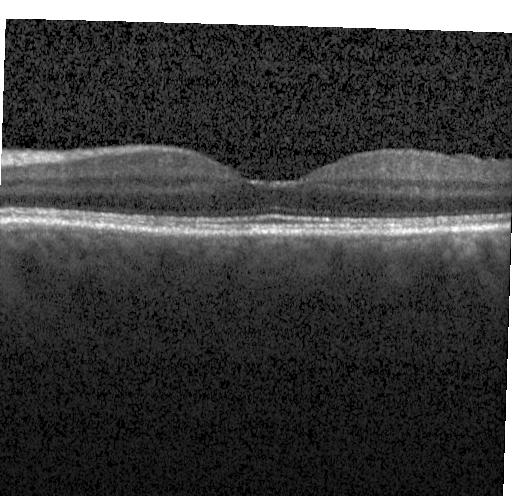 This B-scan demonstrates no evidence of CNV, DME, or drusen.